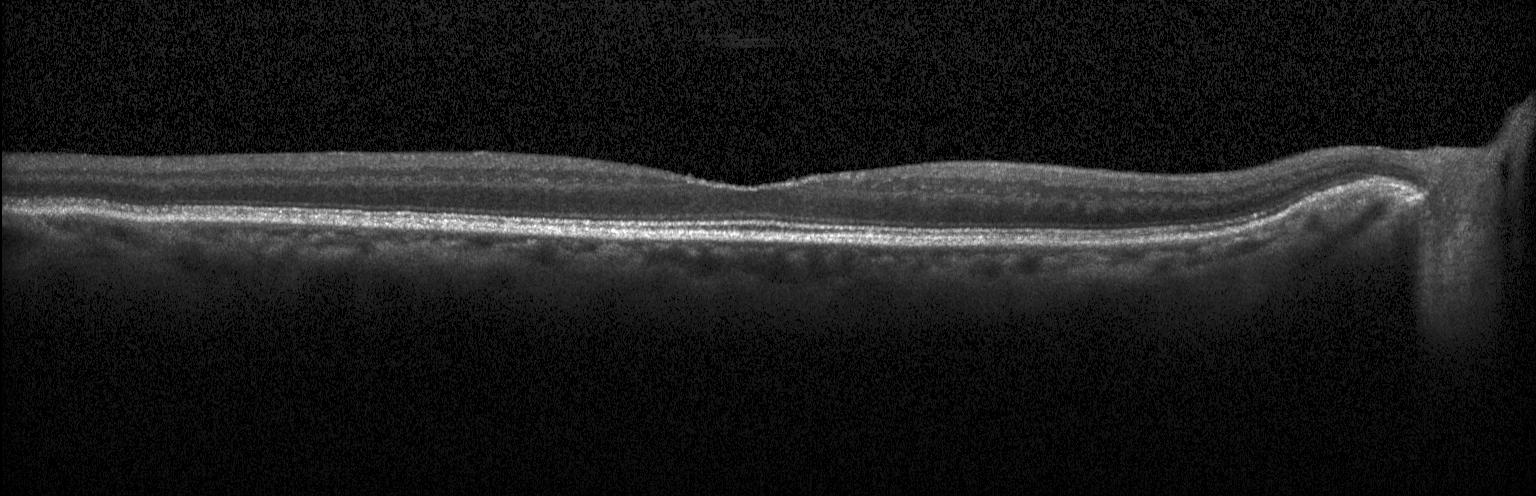
Spectral-domain OCT B-scan: no CNV, DME, or drusen.